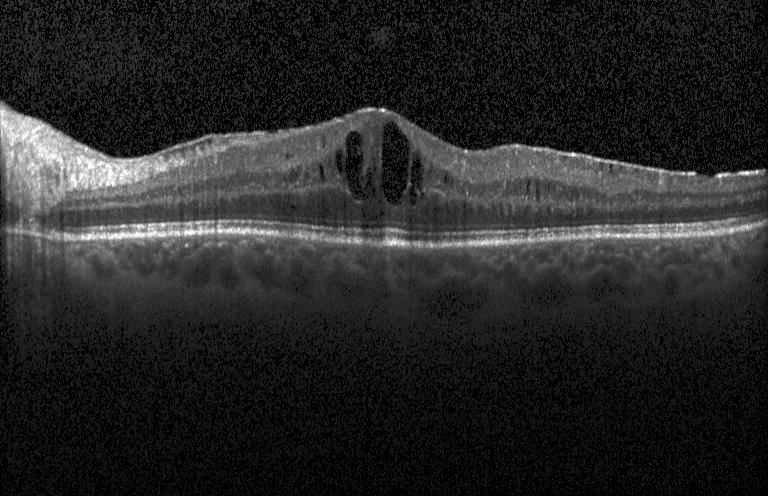
Finding: diabetic macular edema (DME).